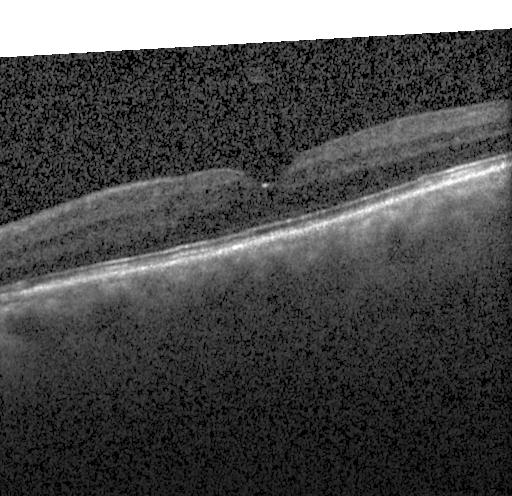
Optical coherence tomography scan
Finding: neither choroidal neovascularization, diabetic macular edema, nor drusen.